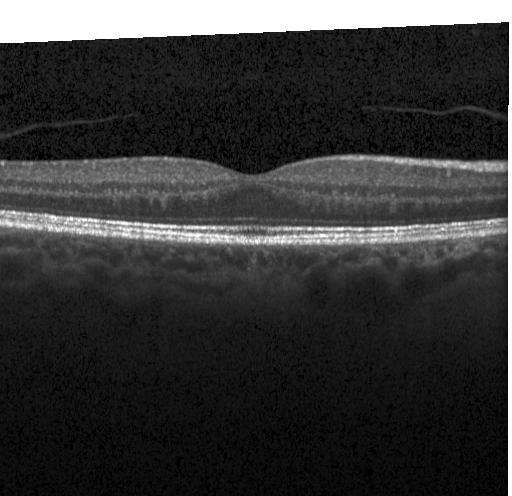
Macular scan; retinal OCT cross-section
Impression: no choroidal neovascularization, no diabetic macular edema, and no drusen.